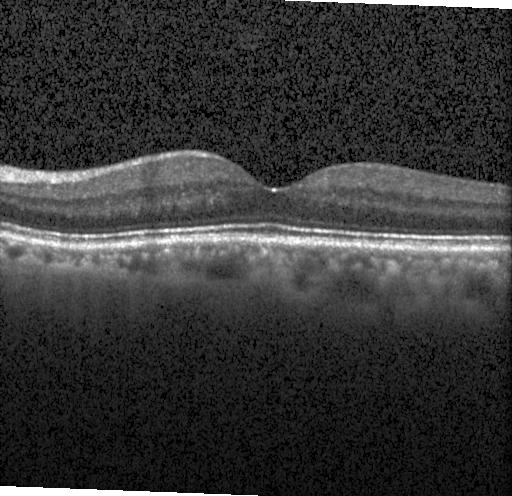

Diagnosis: no evidence of choroidal neovascularization, diabetic macular edema, or drusen.